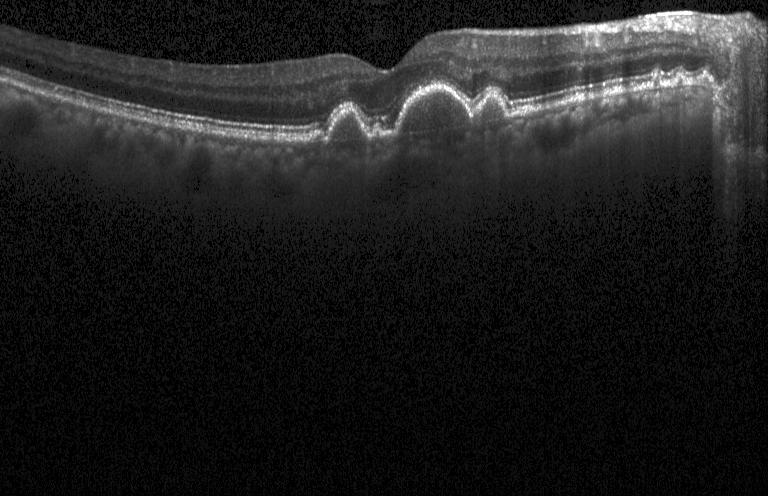
Macular OCT: multiple drusen.